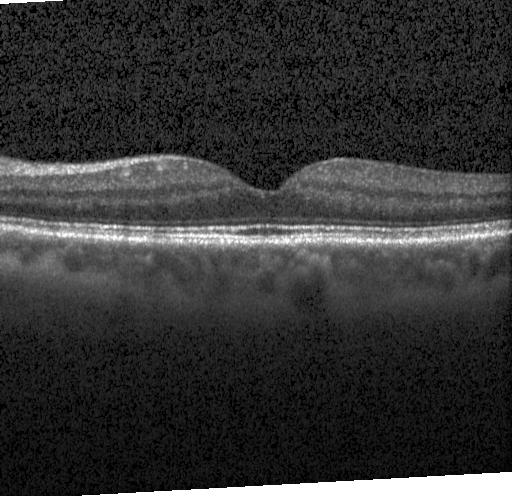 Optical coherence tomography B-scan; instrument: Heidelberg Spectralis; centered on the fovea; spectral-domain optical coherence tomography — Finding: no choroidal neovascularization, no diabetic macular edema, and no drusen.